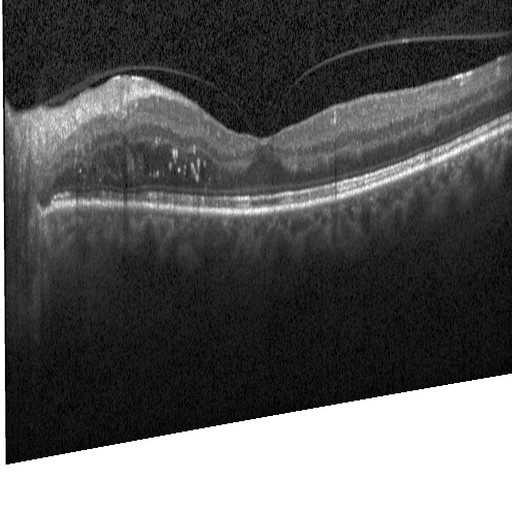
Dx: DME.